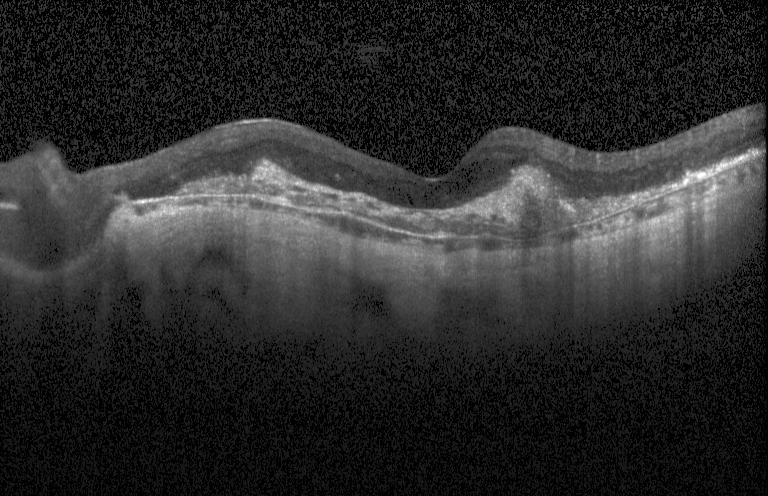

Retinal OCT cross-section. Assessment: a choroidal neovascular membrane.